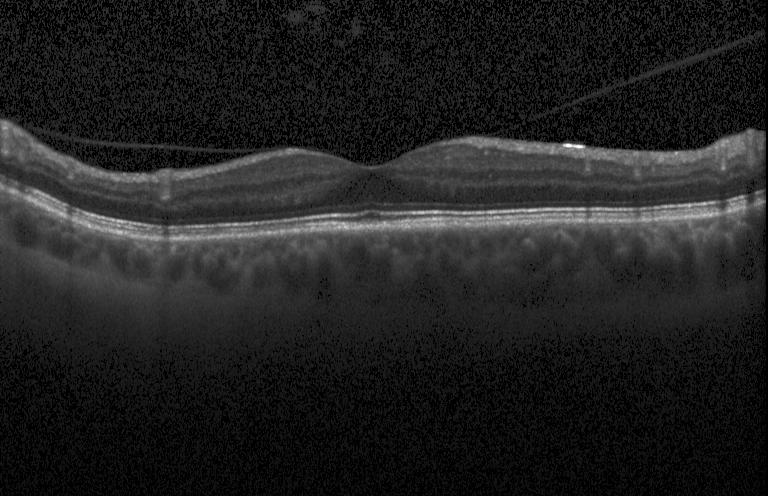 This B-scan demonstrates neither choroidal neovascularization, diabetic macular edema, nor drusen.